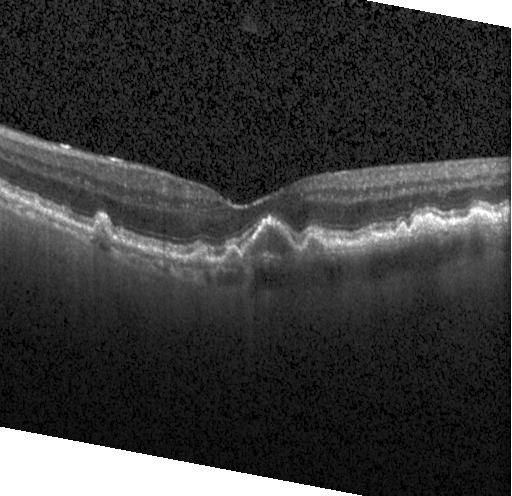 Through the macula; optical coherence tomography B-scan; SD-OCT
Dx: multiple drusen.